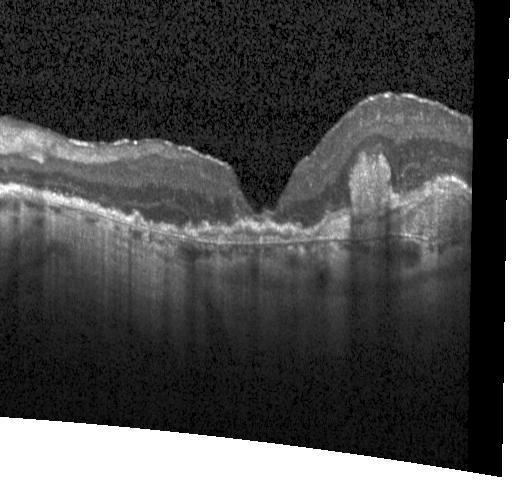

Heidelberg Spectralis · optical coherence tomography scan · centered on the fovea.
Choroidal neovascularization.